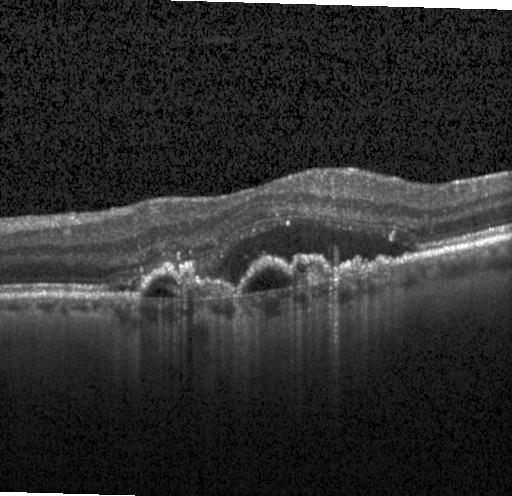

Through the macula, retinal OCT B-scan, spectral-domain optical coherence tomography
Diagnosis: a choroidal neovascular membrane.